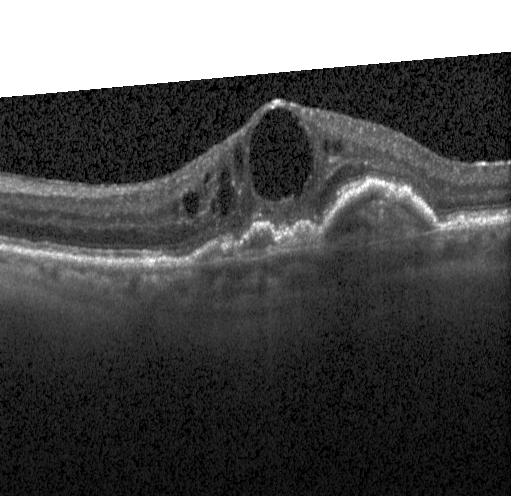
Macular scan; SD-OCT; retinal OCT cross-section; instrument: Heidelberg Spectralis.
Impression: CNV.